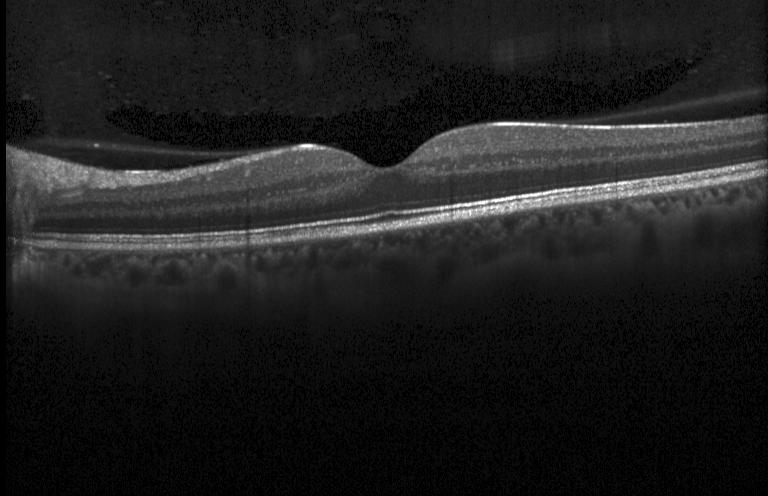

Fovea-centered, instrument: Heidelberg Spectralis, retinal OCT B-scan — Assessment: no evidence of choroidal neovascularization, diabetic macular edema, or drusen.